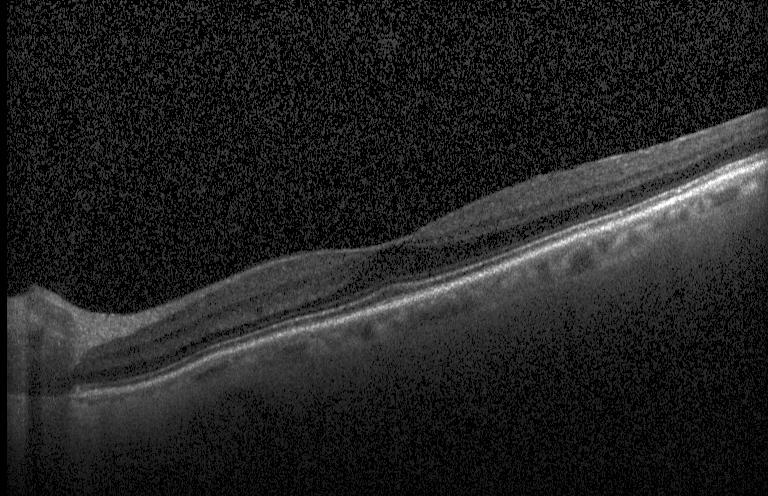 This B-scan demonstrates neither choroidal neovascularization, diabetic macular edema, nor drusen.